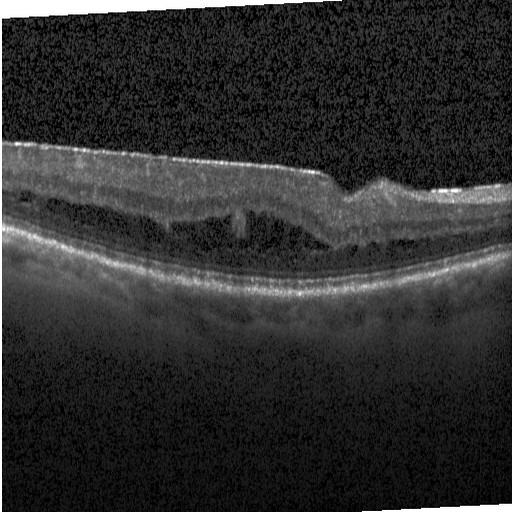 Horizontal scan through the fovea · SD-OCT · Heidelberg Spectralis · retinal OCT cross-section.
Impression: diabetic macular edema.